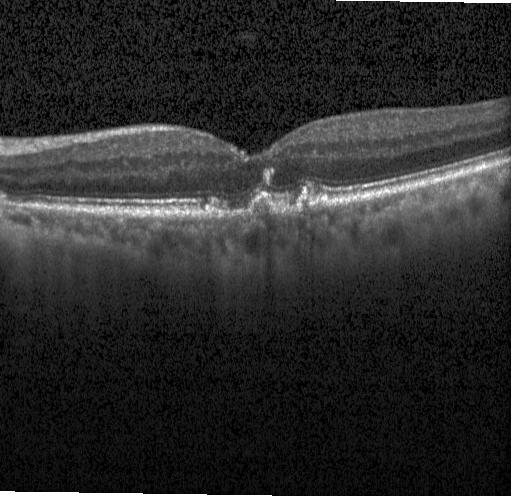
Through the macula; OCT line scan; spectral-domain optical coherence tomography; instrument: Heidelberg Spectralis. The scan shows sub-RPE drusenoid deposits.